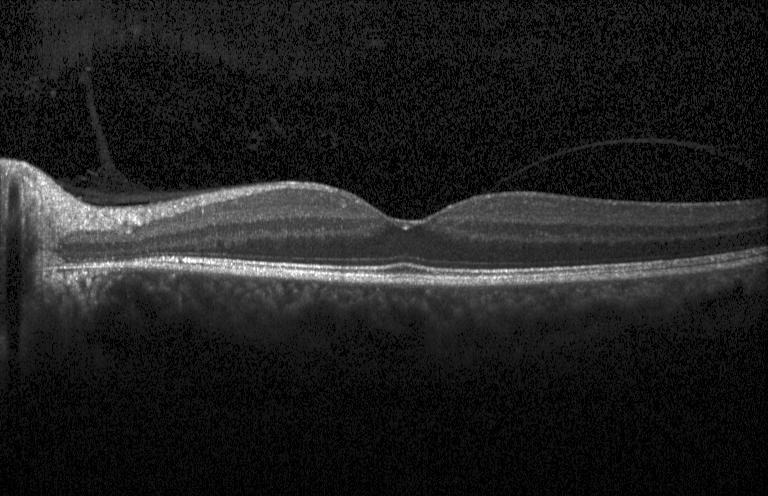
Heidelberg Spectralis, retinal OCT B-scan. No choroidal neovascularization, diabetic macular edema, or drusen.